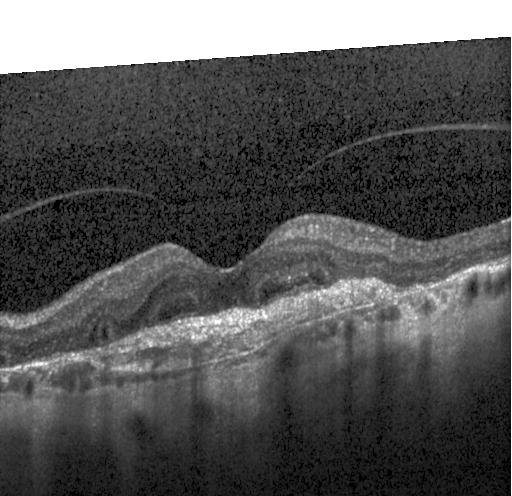 Fovea-centered · retinal OCT B-scan
A choroidal neovascular membrane.